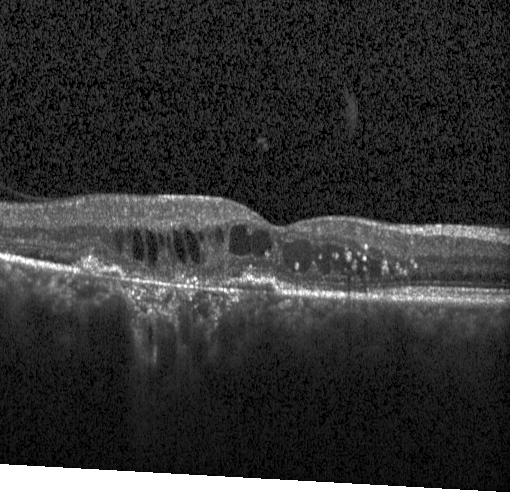
Acquired on a Heidelberg Spectralis · optical coherence tomography B-scan · spectral-domain optical coherence tomography · horizontal scan through the fovea. Dx: choroidal neovascularization.